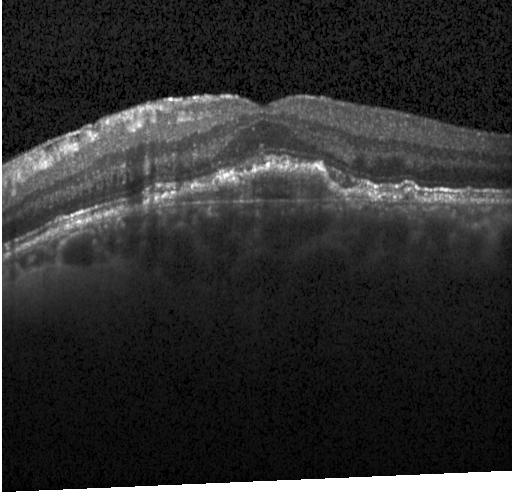 Spectral-domain OCT · retinal OCT B-scan · macular scan · instrument: Heidelberg Spectralis
Impression: CNV.